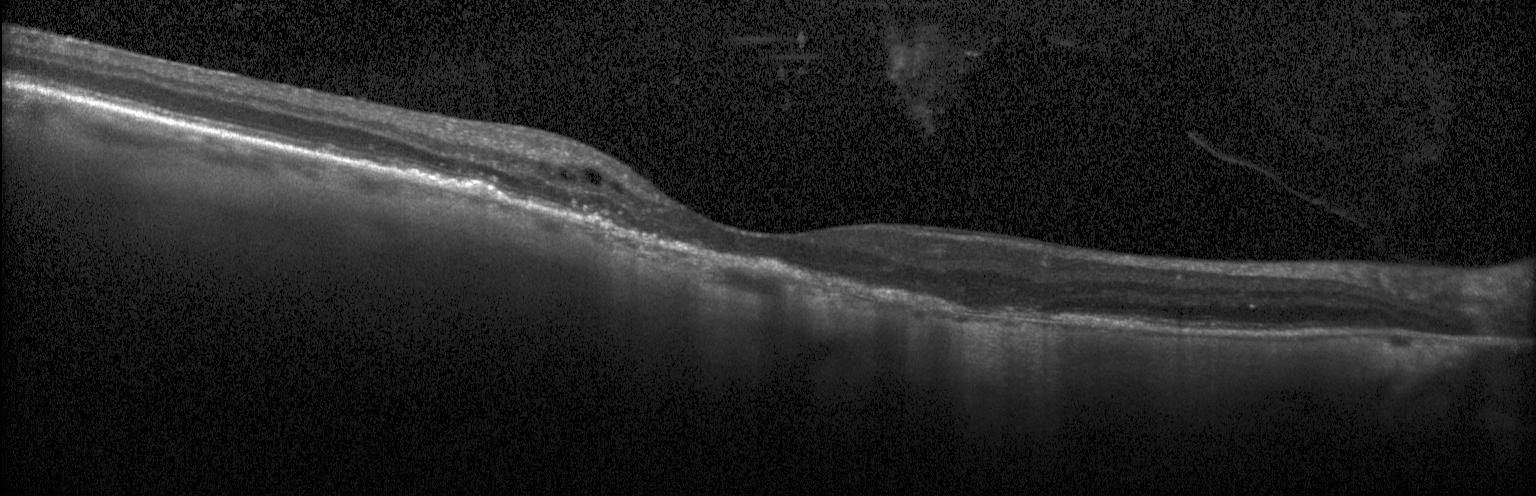

Spectral-domain OCT; Heidelberg Spectralis OCT system; centered on the fovea; retinal OCT B-scan.
Finding: a choroidal neovascular membrane.